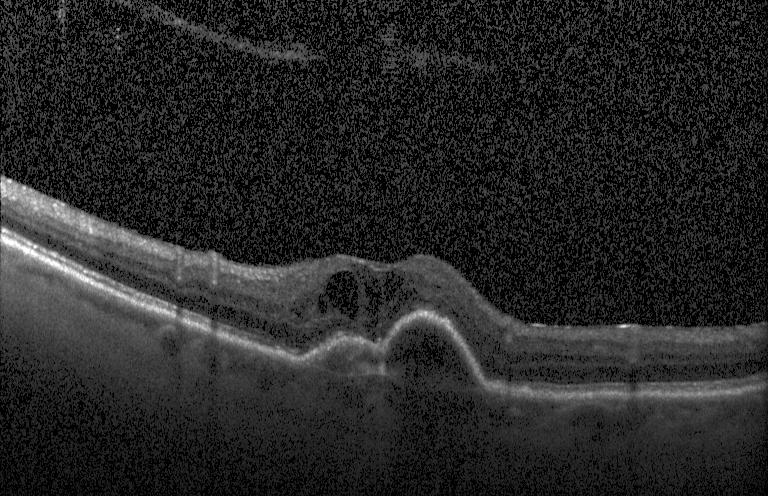 Heidelberg Spectralis, centered on the fovea, spectral-domain optical coherence tomography, retinal OCT cross-section — This B-scan demonstrates choroidal neovascularization.